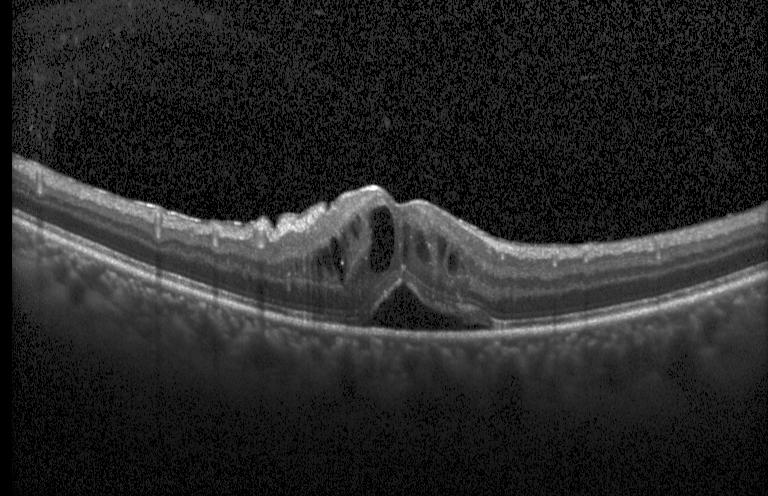

Finding: diabetic macular edema (DME).